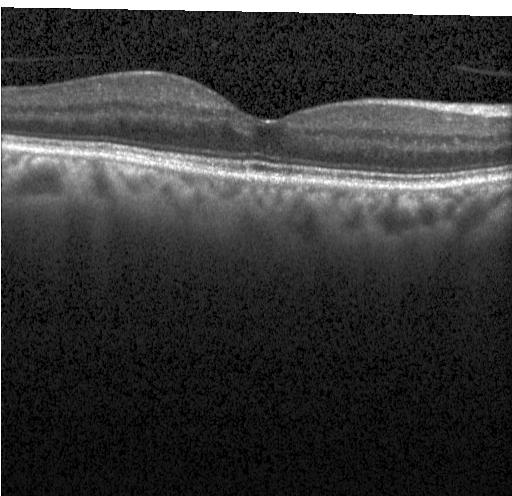 Optical coherence tomography B-scan. Macular OCT: no evidence of CNV, DME, or drusen.